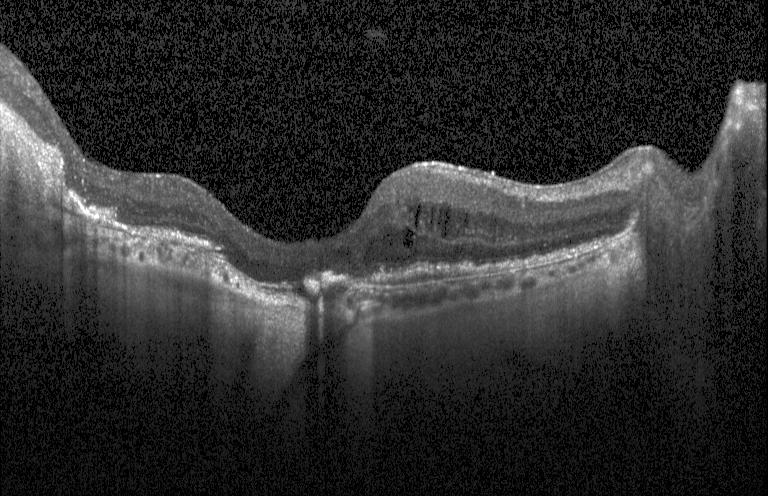 Retinal OCT cross-section. Spectral-domain optical coherence tomography.
This B-scan demonstrates CNV.